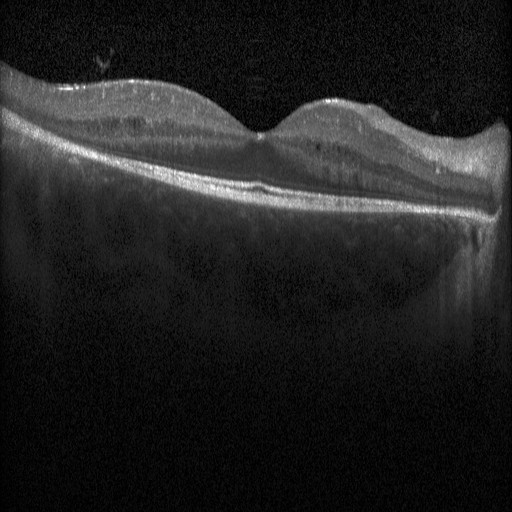 Impression: diabetic macular edema.